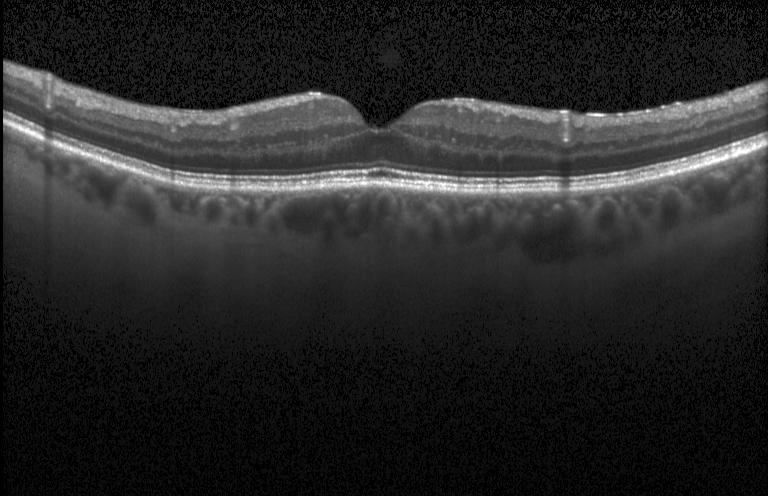 Horizontal scan through the fovea, OCT B-scan
Finding: no choroidal neovascularization, diabetic macular edema, or drusen.